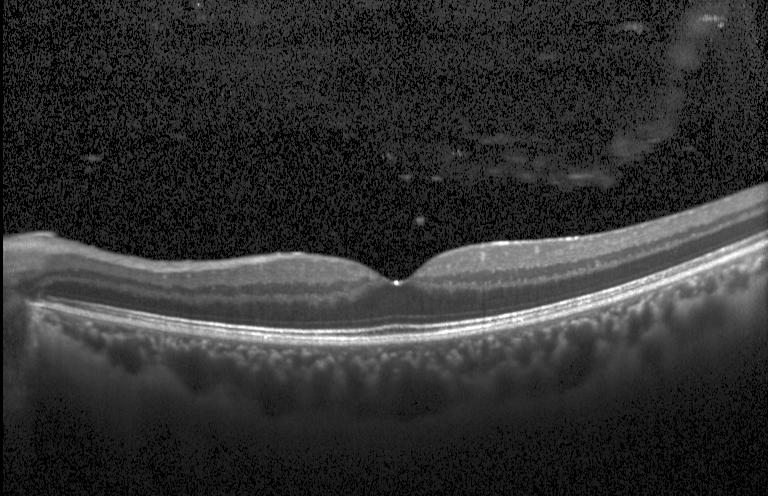
Finding: no choroidal neovascularization, no diabetic macular edema, and no drusen.